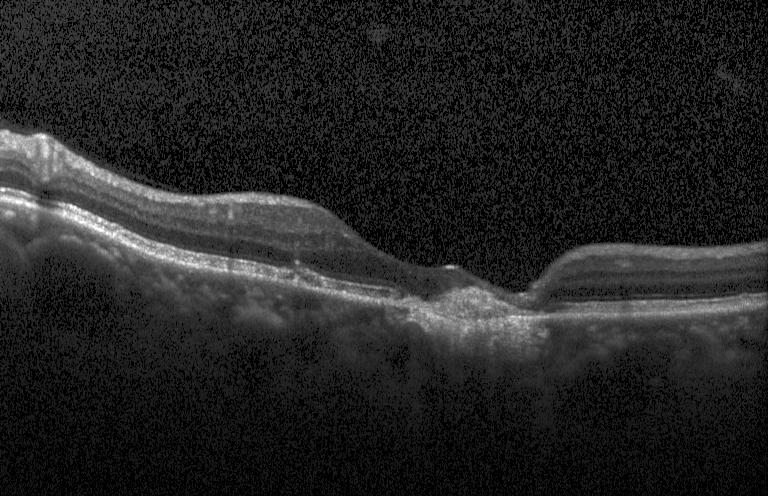 A choroidal neovascular membrane.